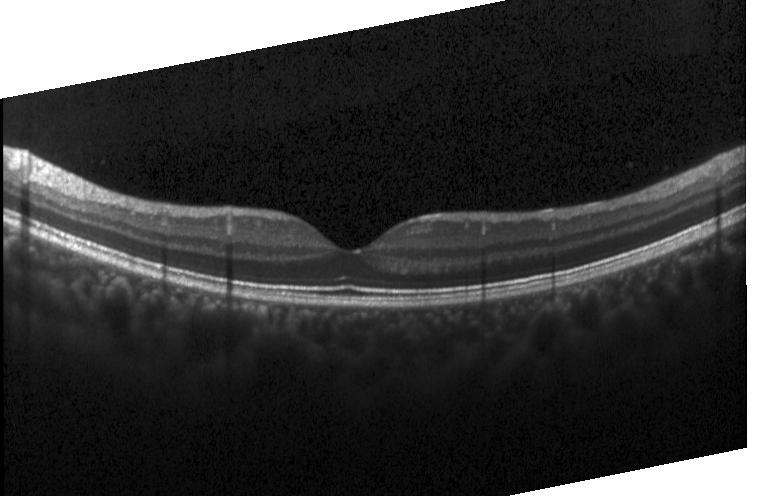
Retinal OCT cross-section showing no choroidal neovascularization, no diabetic macular edema, and no drusen.